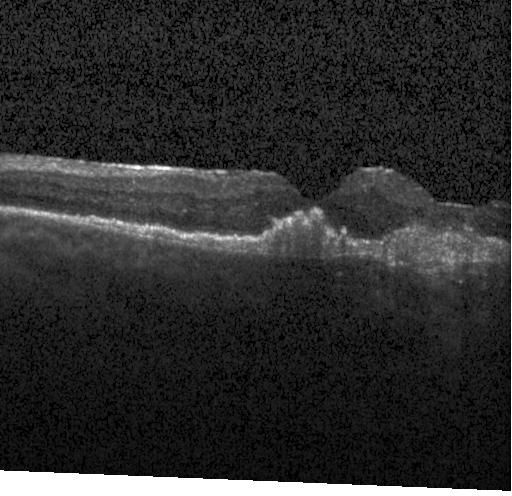 Heidelberg Spectralis OCT system; OCT B-scan; centered on the fovea; SD-OCT. OCT finding: a choroidal neovascular membrane.